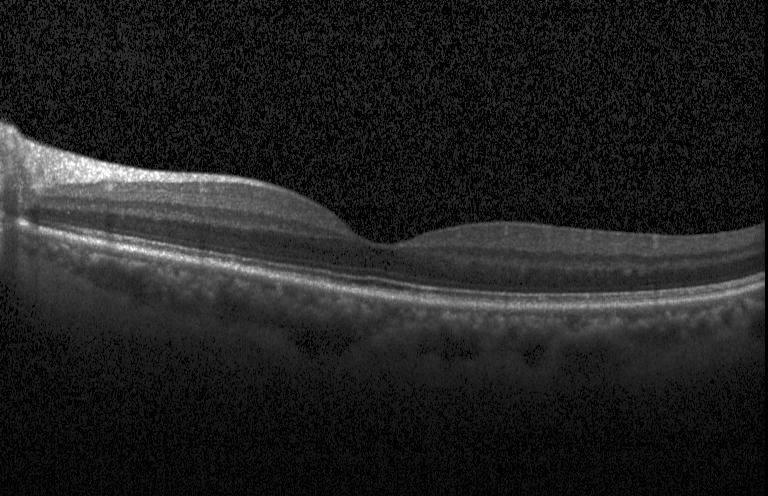
Spectral-domain optical coherence tomography; retinal OCT B-scan — Diagnosis: no evidence of choroidal neovascularization, diabetic macular edema, or drusen.